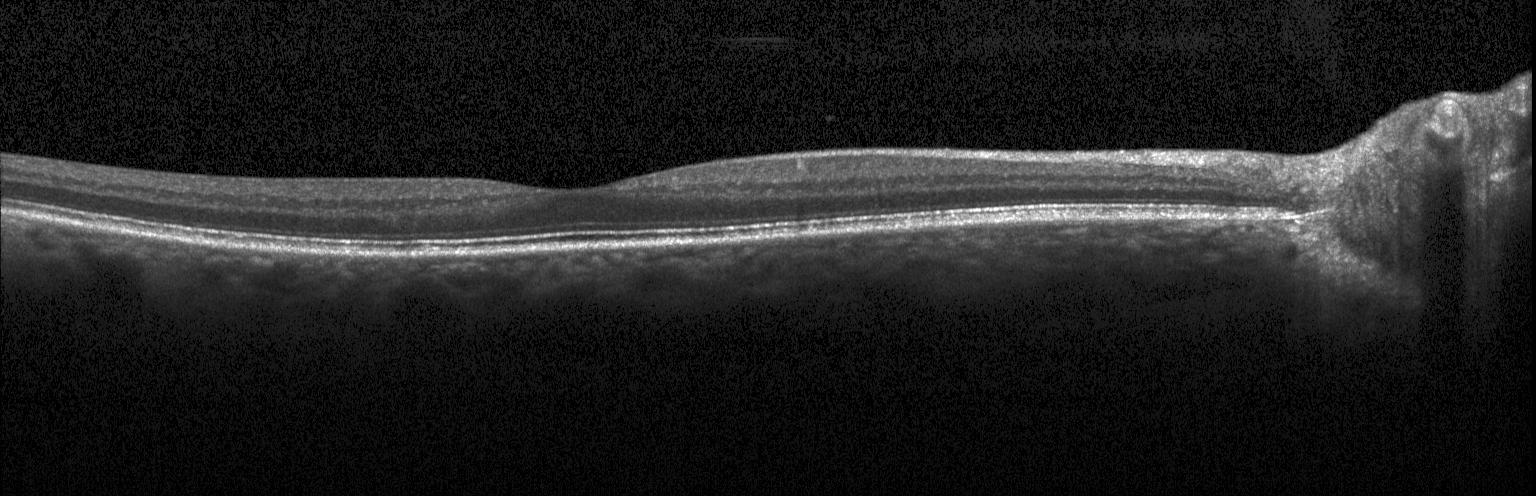 Heidelberg Spectralis. Spectral-domain OCT. Retinal OCT B-scan.
Diagnosis: no choroidal neovascularization, diabetic macular edema, or drusen.